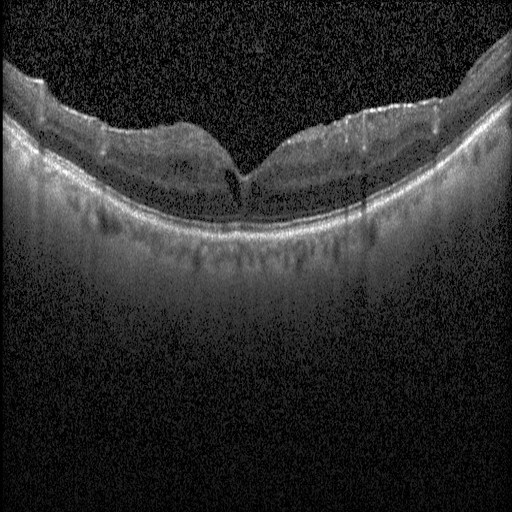 Spectral-domain OCT · Heidelberg Spectralis · optical coherence tomography B-scan · macular scan — Finding: DME.